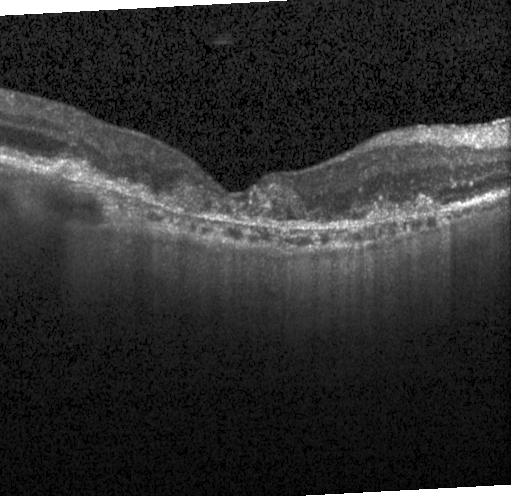
Finding: a choroidal neovascular membrane.